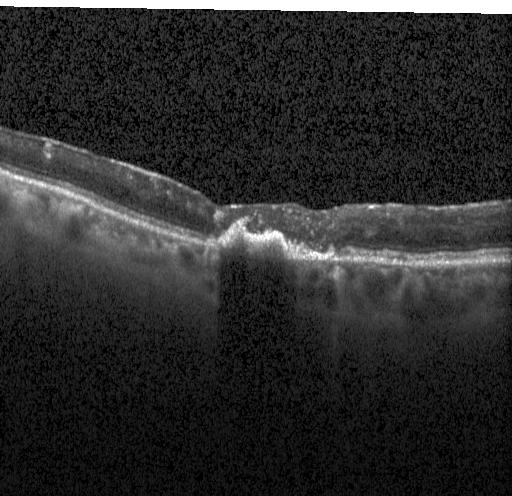
Retinal OCT cross-section · horizontal scan through the fovea · Heidelberg Spectralis OCT system · SD-OCT.
Finding: CNV.